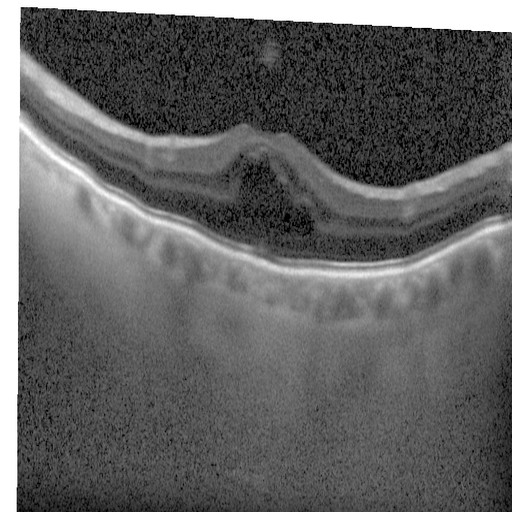 Diagnosis: DME.